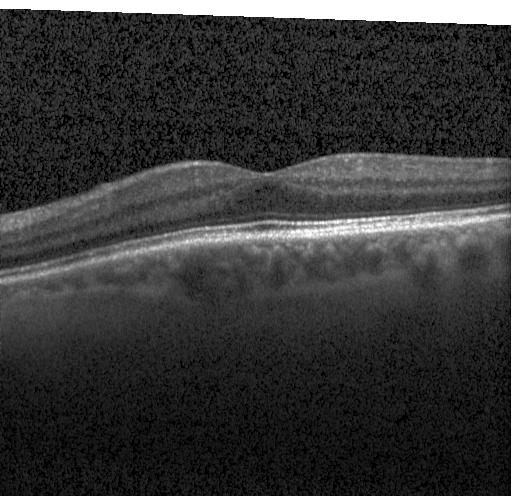 Spectral-domain OCT, retinal OCT cross-section, instrument: Heidelberg Spectralis.
Impression: neither choroidal neovascularization, diabetic macular edema, nor drusen.